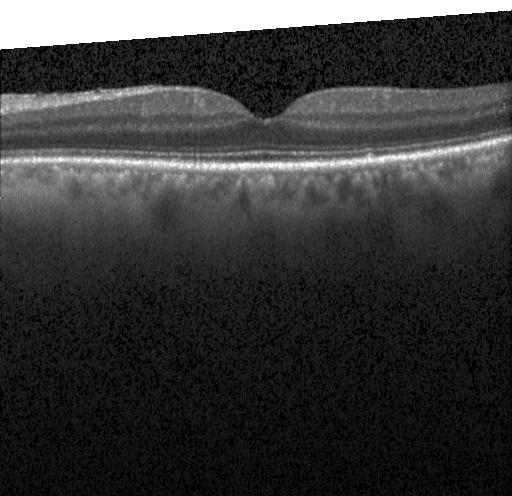
Spectral-domain OCT B-scan: no choroidal neovascularization, diabetic macular edema, or drusen.